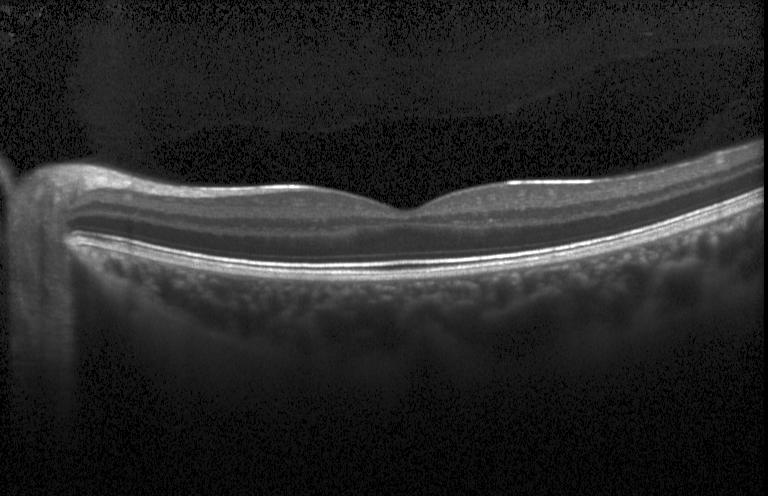

Retinal OCT cross-section.
Dx: no choroidal neovascularization, diabetic macular edema, or drusen.